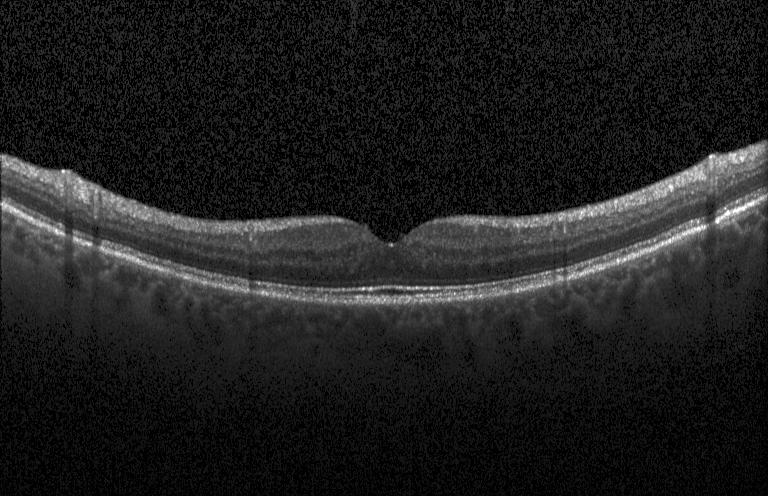

Optical coherence tomography B-scan
This B-scan demonstrates no CNV, DME, or drusen.